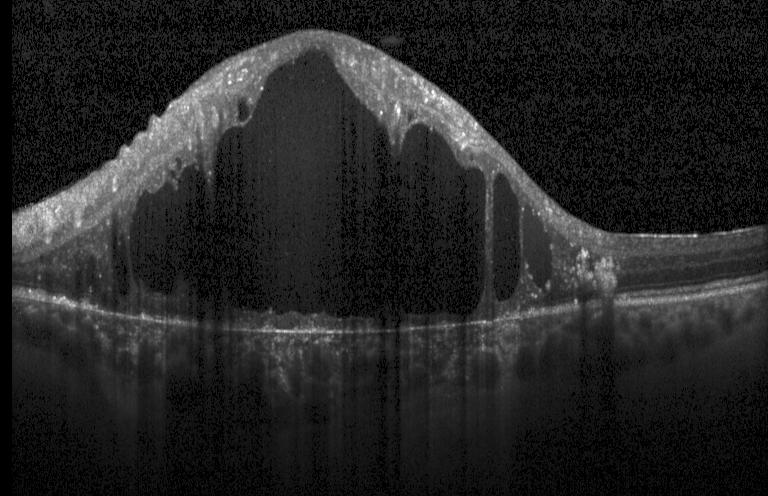

Finding: DME.